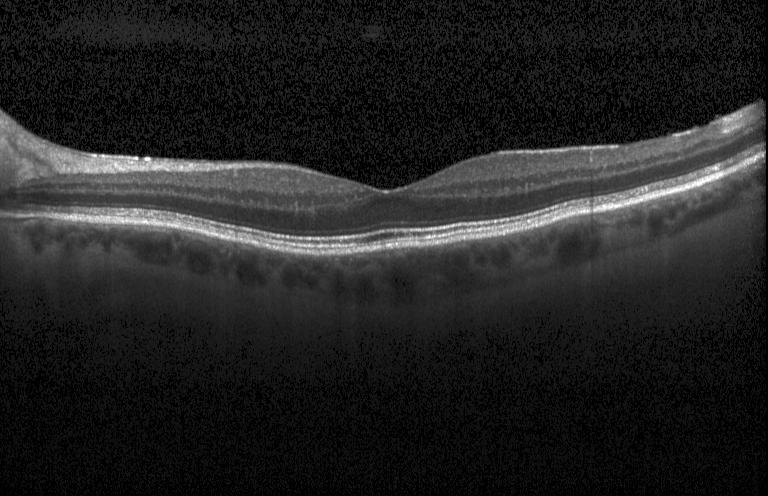
OCT line scan; Heidelberg Spectralis OCT system; spectral-domain OCT; macular scan — Finding: no choroidal neovascularization, no diabetic macular edema, and no drusen.